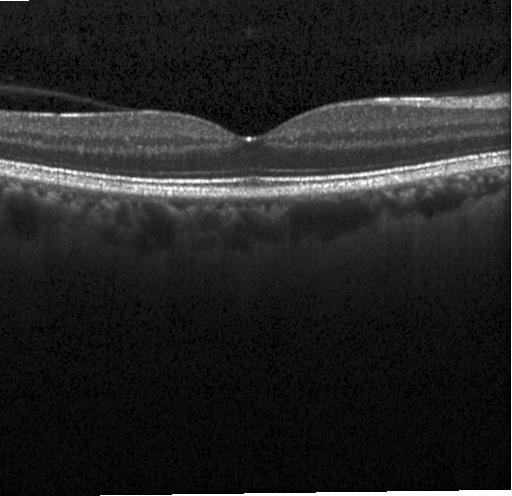
Diagnosis: neither choroidal neovascularization, diabetic macular edema, nor drusen.